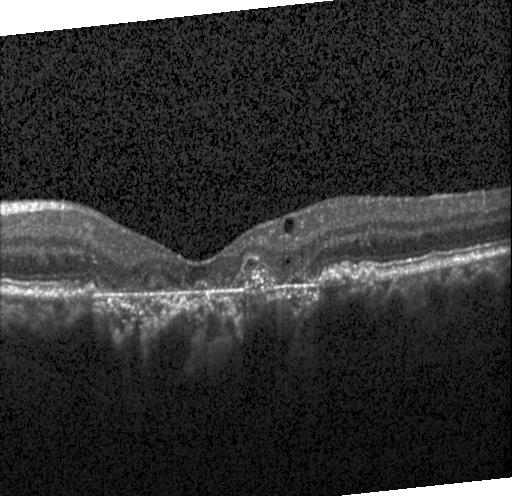
Retinal OCT cross-section
Dx: a choroidal neovascular membrane.